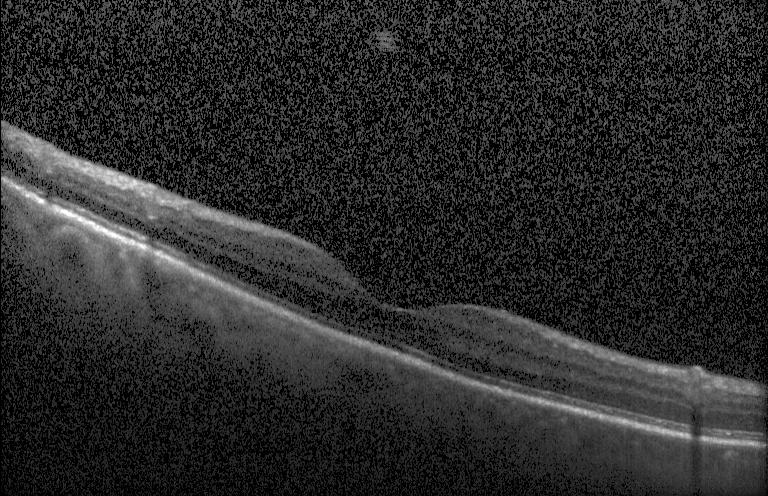
Finding: no evidence of choroidal neovascularization, diabetic macular edema, or drusen.